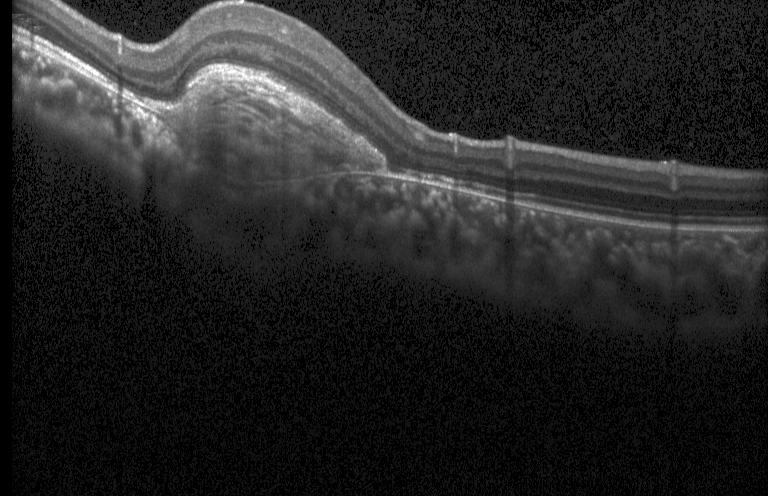

Spectral-domain optical coherence tomography. Heidelberg Spectralis OCT system. OCT line scan. Centered on the fovea. OCT finding: CNV.